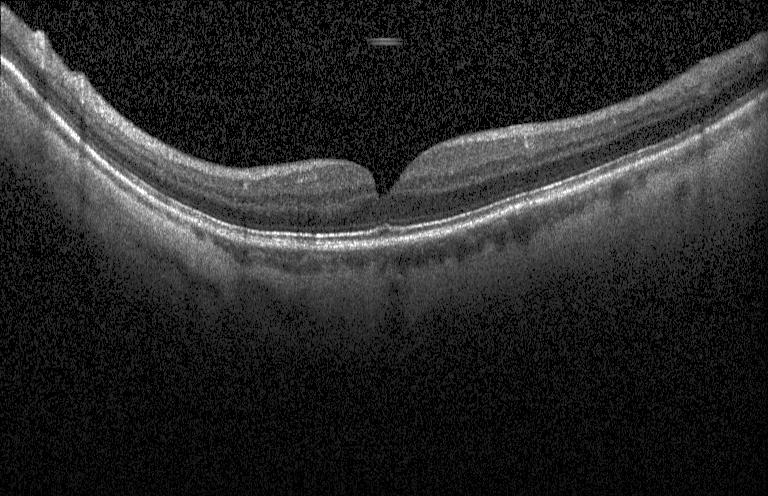

Diagnosis: no choroidal neovascularization, diabetic macular edema, or drusen.